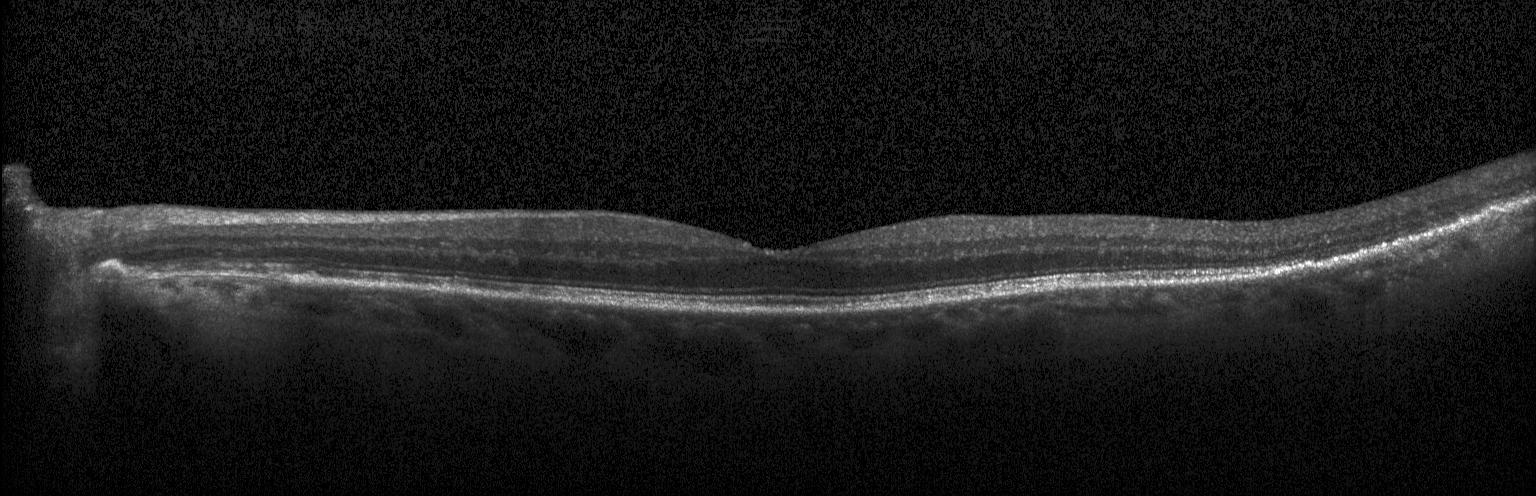
Heidelberg Spectralis · spectral-domain OCT · optical coherence tomography B-scan · centered on the fovea. This B-scan demonstrates no CNV, no DME, and no drusen.